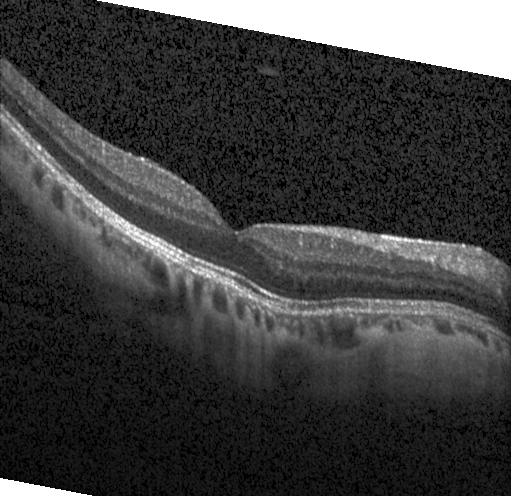
OCT line scan. Finding: neither choroidal neovascularization, diabetic macular edema, nor drusen.